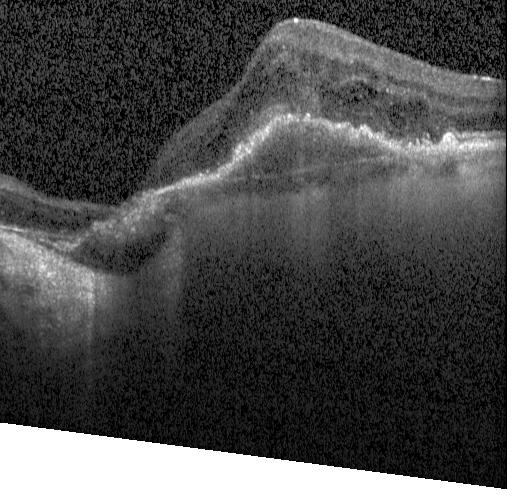
Spectral-domain OCT · centered on the fovea · OCT B-scan. This B-scan demonstrates choroidal neovascularization (CNV).